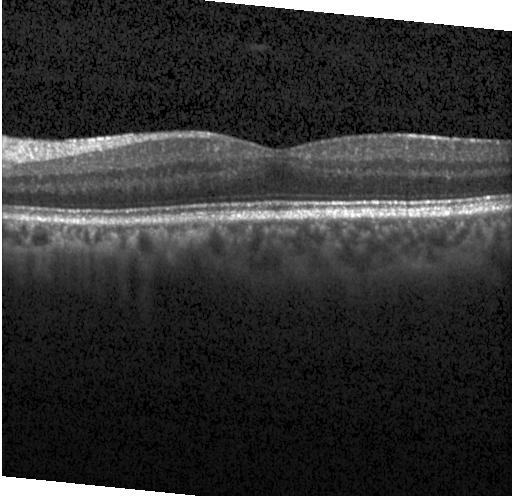 Retinal OCT B-scan · fovea-centered · instrument: Heidelberg Spectralis.
Diagnosis: no CNV, no DME, and no drusen.